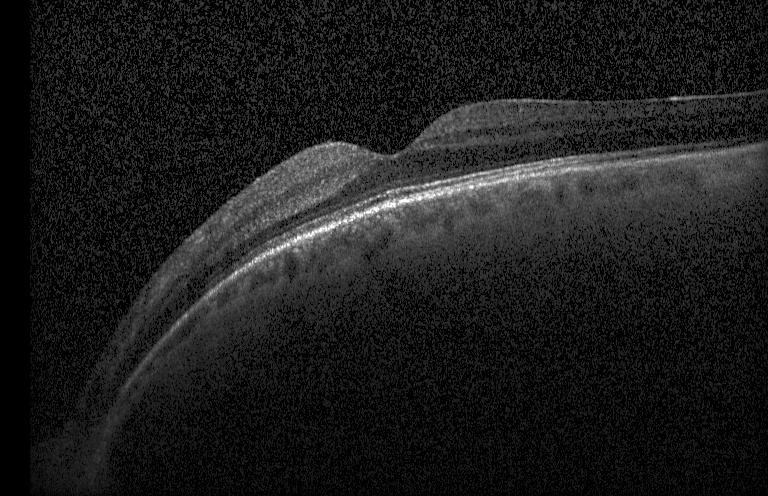

Retinal OCT cross-section · spectral-domain optical coherence tomography. Impression: neither choroidal neovascularization, diabetic macular edema, nor drusen.